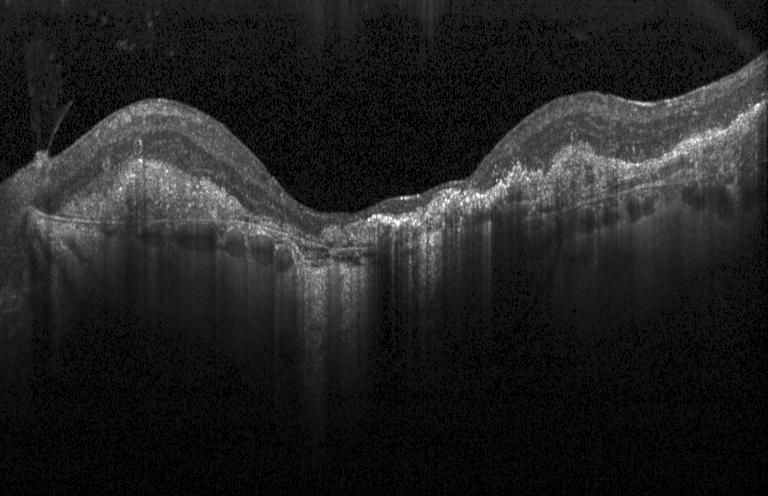

Finding: a choroidal neovascular membrane.